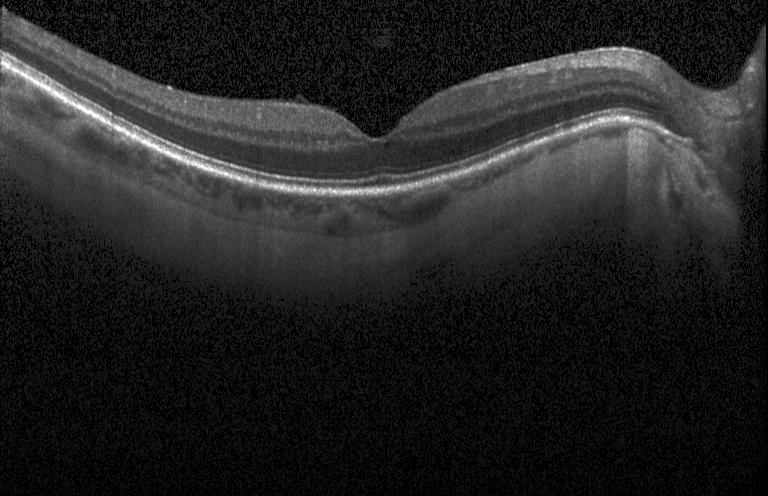 Heidelberg Spectralis · optical coherence tomography scan · horizontal scan through the fovea · spectral-domain optical coherence tomography. Impression: no evidence of choroidal neovascularization, diabetic macular edema, or drusen.